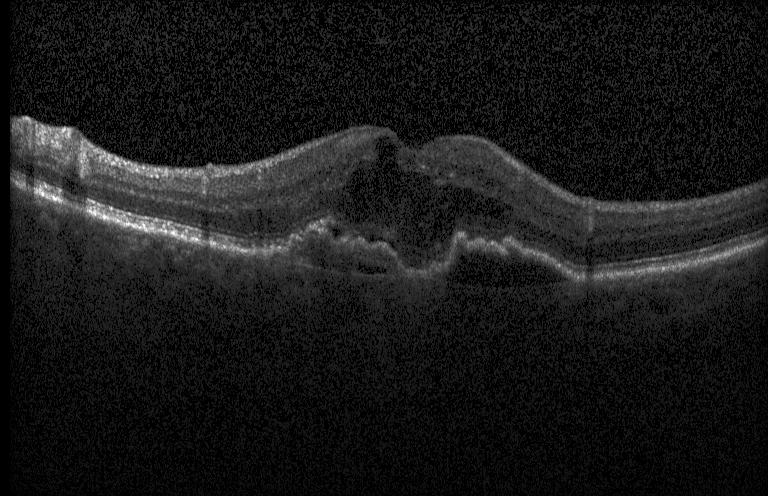

Dx: CNV.